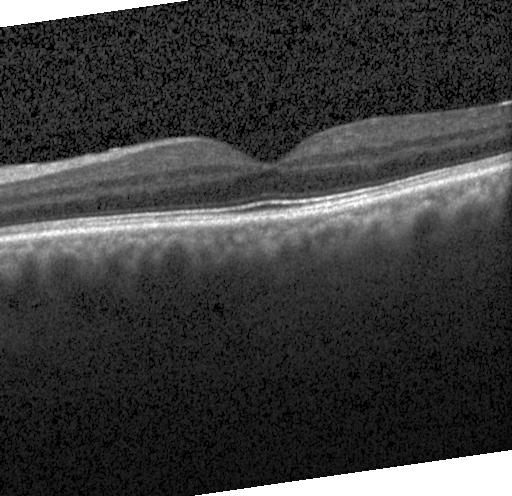
Assessment: no evidence of choroidal neovascularization, diabetic macular edema, or drusen.